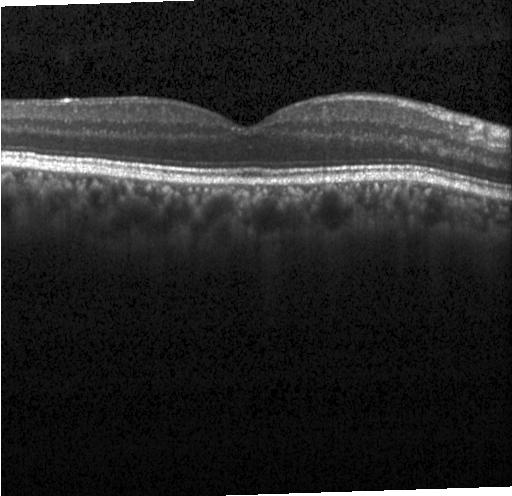 Retinal OCT B-scan.
Impression: no CNV, no DME, and no drusen.